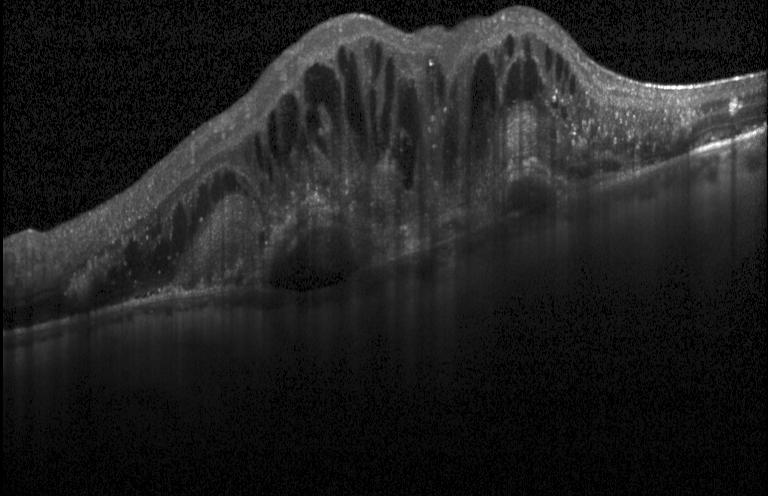
Macular scan, retinal OCT cross-section, SD-OCT, instrument: Heidelberg Spectralis. Diagnosis: choroidal neovascularization.